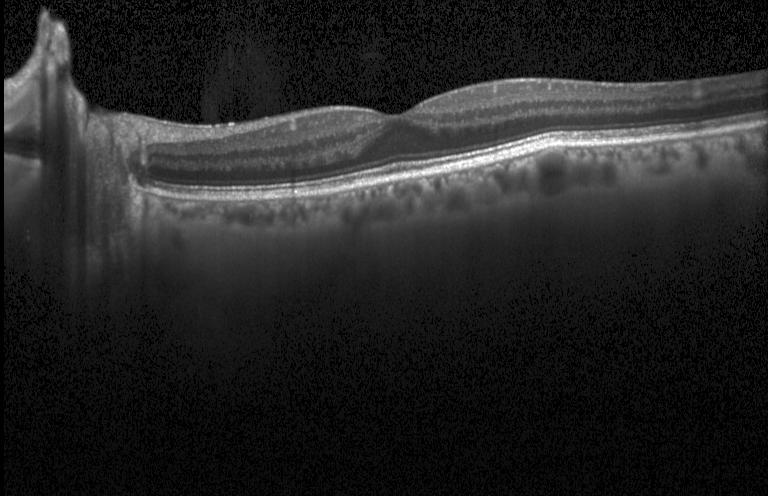
OCT B-scan. Horizontal scan through the fovea
Impression: no evidence of choroidal neovascularization, diabetic macular edema, or drusen.